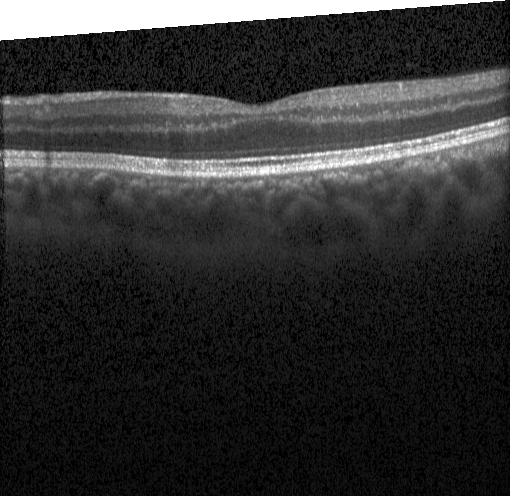 OCT B-scan. Spectral-domain OCT. Horizontal scan through the fovea. Heidelberg Spectralis OCT system — No choroidal neovascularization, diabetic macular edema, or drusen.